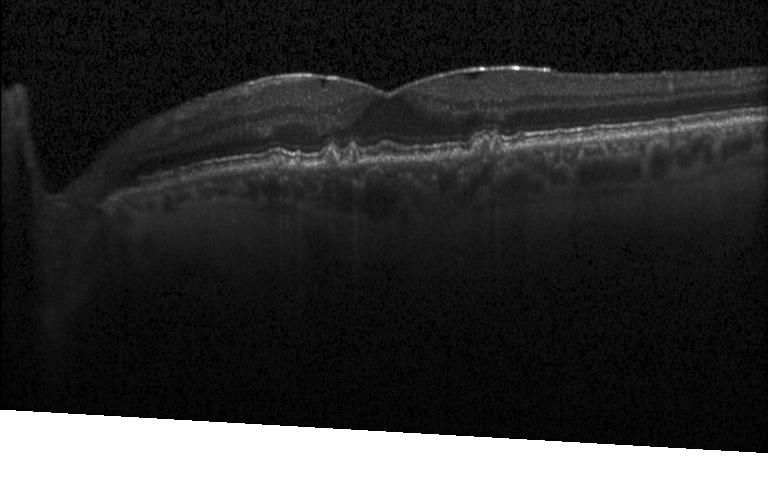

Macular OCT demonstrating drusen.